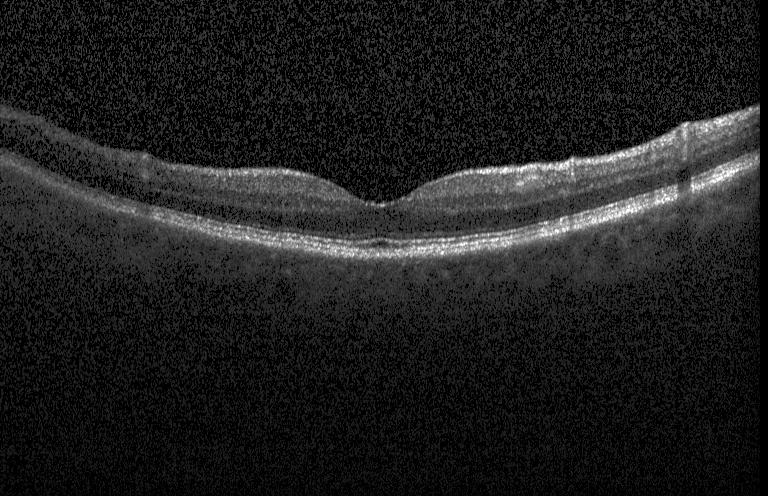

SD-OCT · Heidelberg Spectralis OCT system · macular scan · OCT line scan
Impression: no choroidal neovascularization, diabetic macular edema, or drusen.